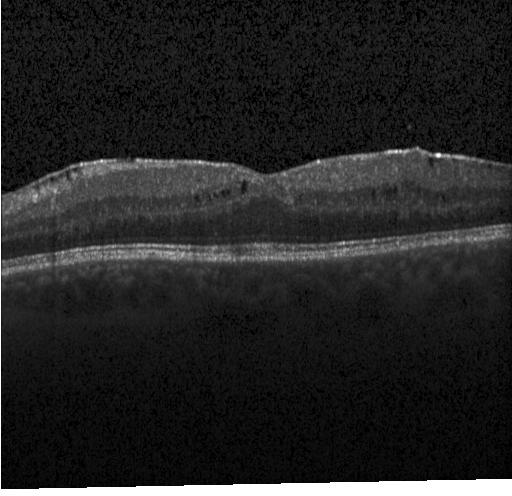

Spectral-domain optical coherence tomography. Optical coherence tomography B-scan. Heidelberg Spectralis OCT system
Finding: DME.